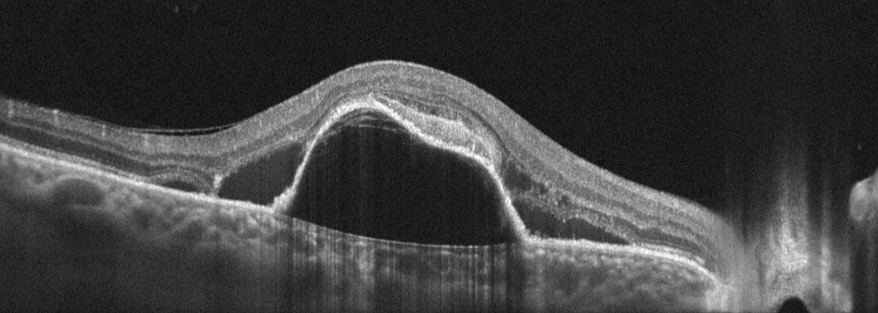
Diagnosis: age-related macular degeneration.